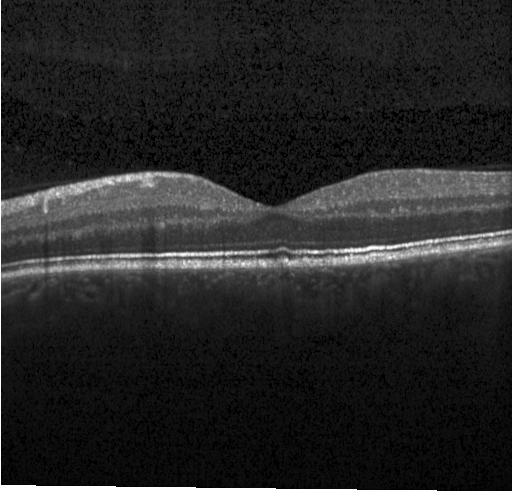

Retinal OCT cross-section showing sub-RPE drusenoid deposits.